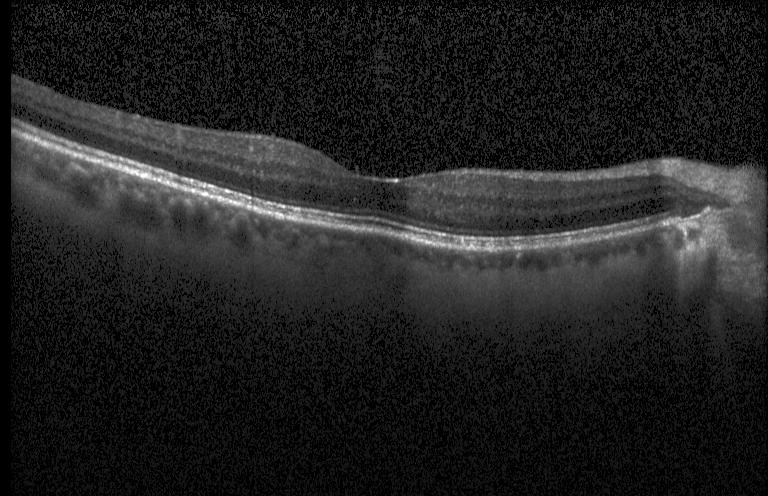
Through the macula, optical coherence tomography B-scan, spectral-domain OCT — Impression: no evidence of choroidal neovascularization, diabetic macular edema, or drusen.